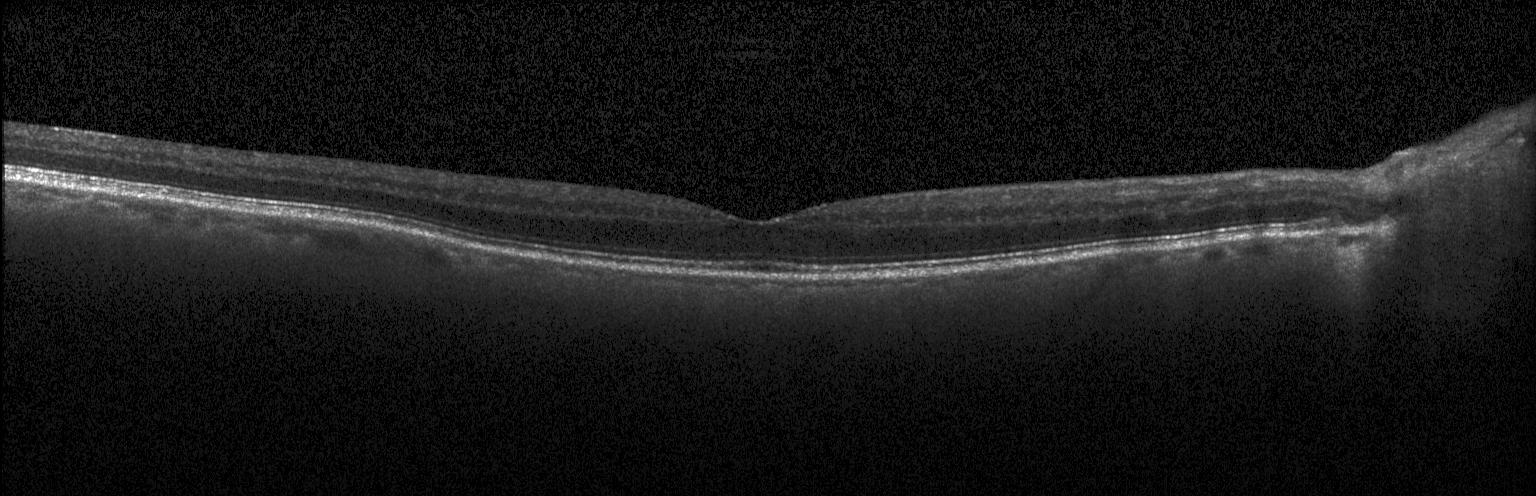

OCT B-scan showing no choroidal neovascularization, no diabetic macular edema, and no drusen.